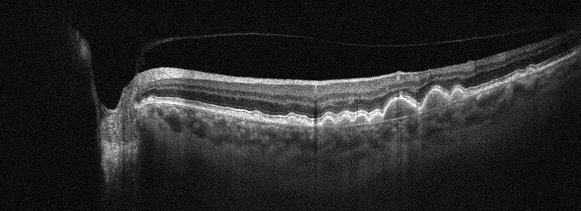

Retinal OCT B-scan. Macular OCT: AMD.